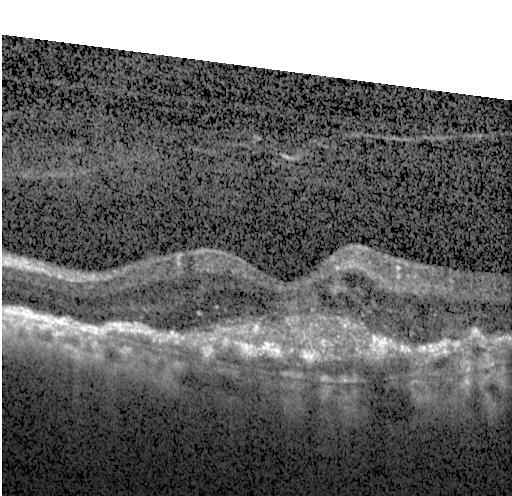
Retinal OCT B-scan. Heidelberg Spectralis OCT system. Fovea-centered.
Macular OCT: a choroidal neovascular membrane.